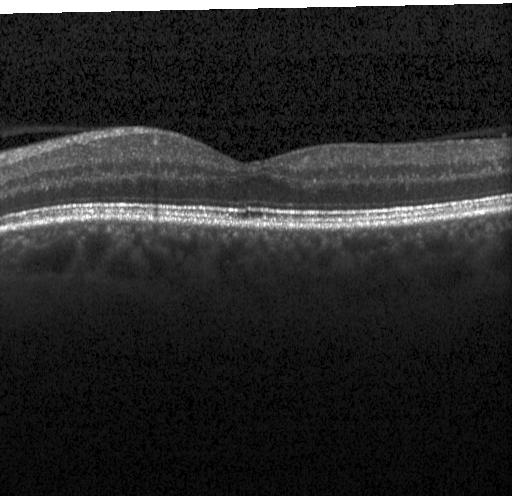
Diagnosis: neither choroidal neovascularization, diabetic macular edema, nor drusen.